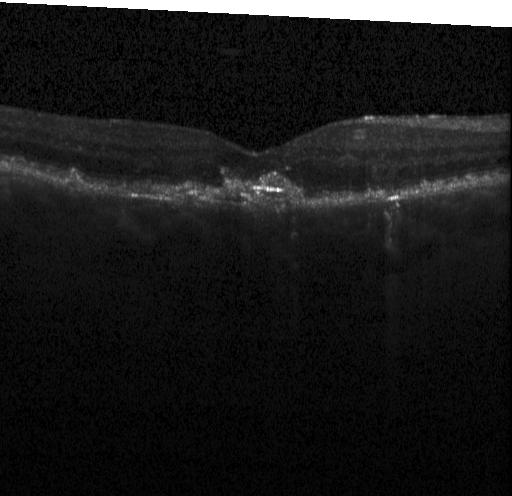

SD-OCT, optical coherence tomography scan, Heidelberg Spectralis. Diagnosis: a choroidal neovascular membrane.